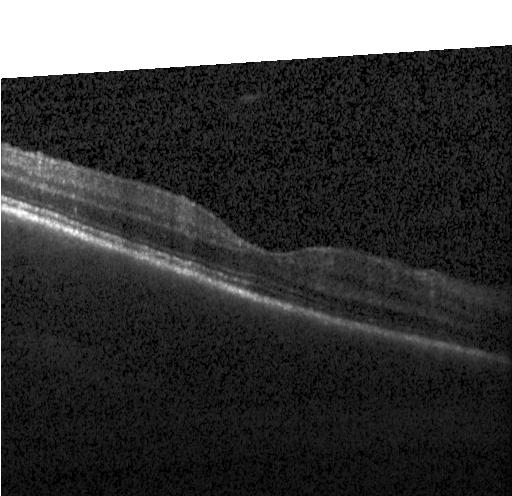

OCT B-scan; through the macula.
The scan shows no choroidal neovascularization, no diabetic macular edema, and no drusen.